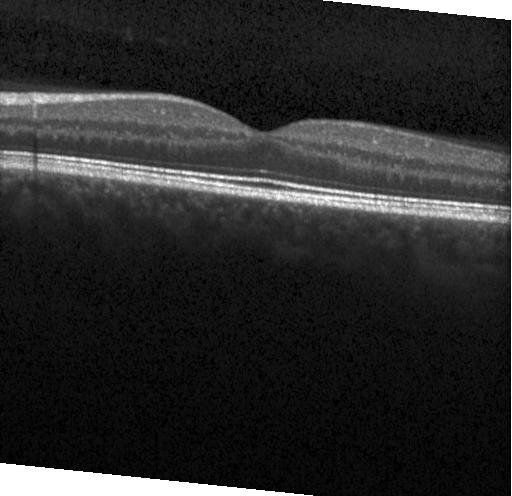 Horizontal scan through the fovea; OCT line scan
Diagnosis: no choroidal neovascularization, diabetic macular edema, or drusen.